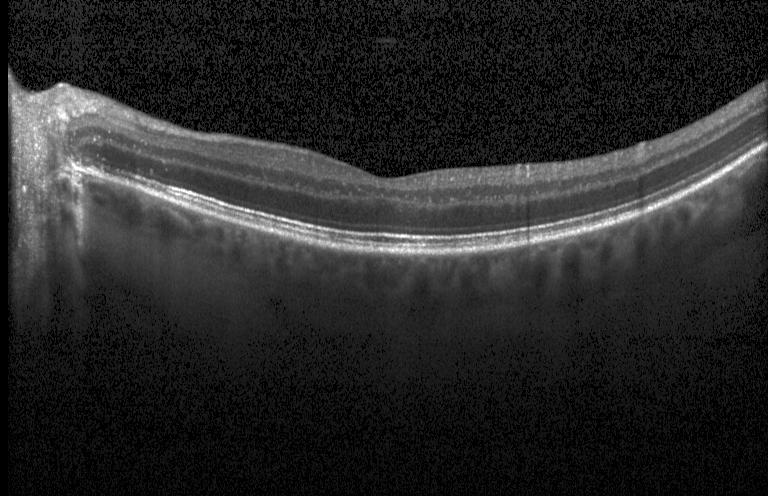

SD-OCT. Retinal OCT cross-section. Assessment: no choroidal neovascularization, diabetic macular edema, or drusen.